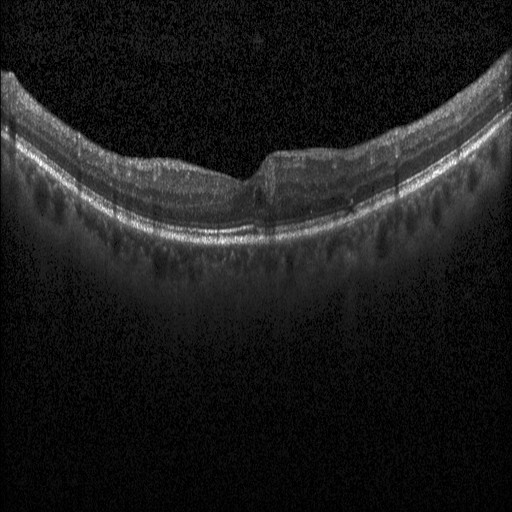

Macular OCT demonstrating diabetic macular edema.